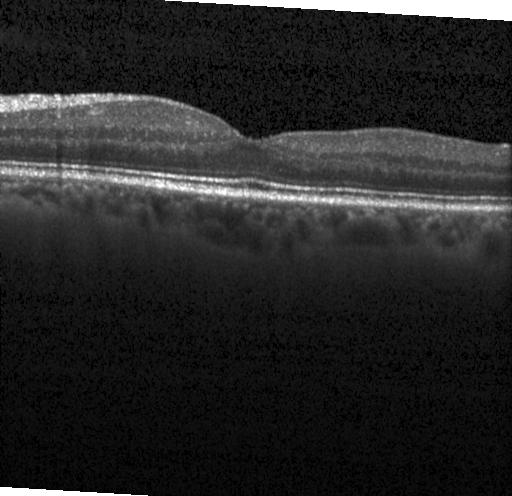

Spectral-domain OCT; optical coherence tomography scan; horizontal scan through the fovea; instrument: Heidelberg Spectralis — The scan shows no CNV, DME, or drusen.